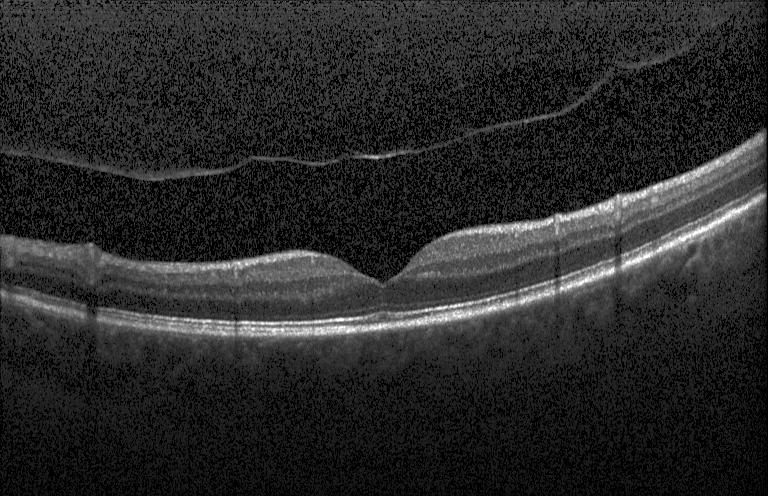 Macular OCT: neither choroidal neovascularization, diabetic macular edema, nor drusen.